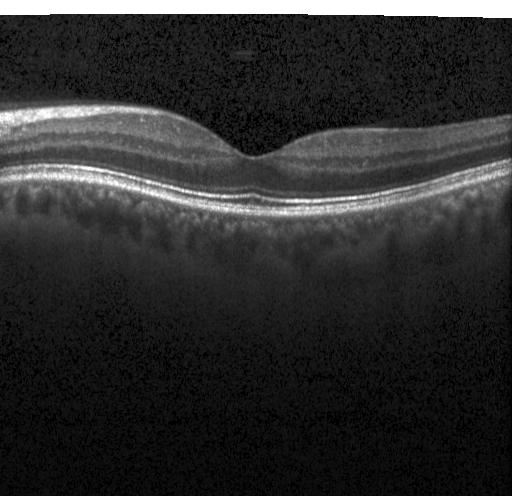

Optical coherence tomography B-scan.
Macular OCT: neither choroidal neovascularization, diabetic macular edema, nor drusen.